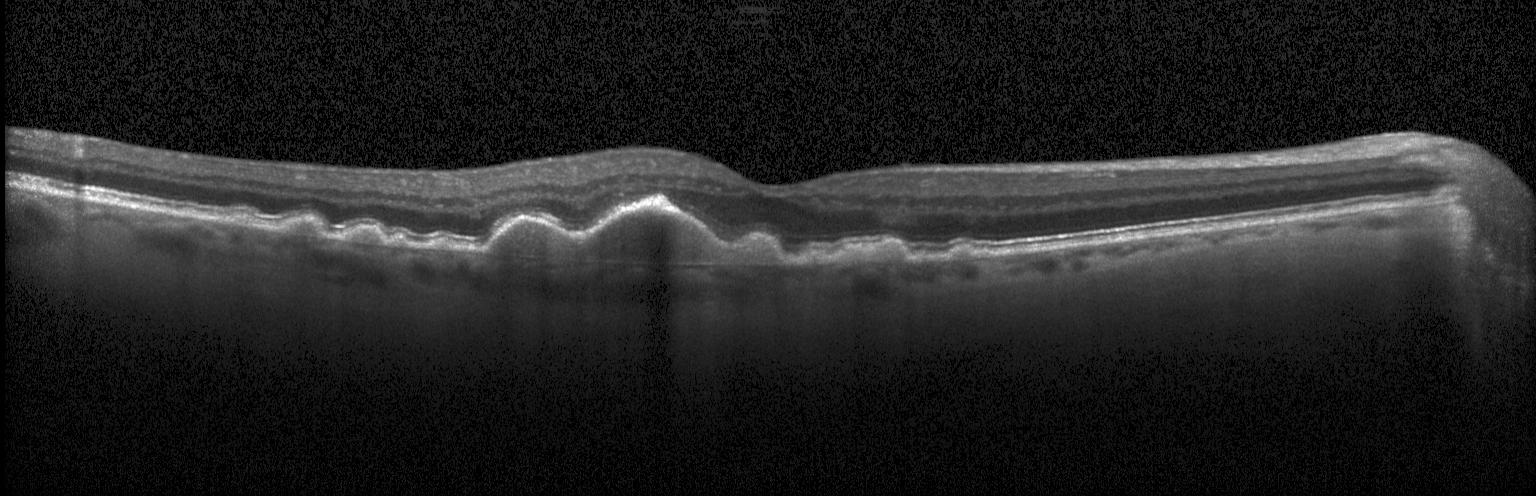
Diagnosis: a choroidal neovascular membrane.